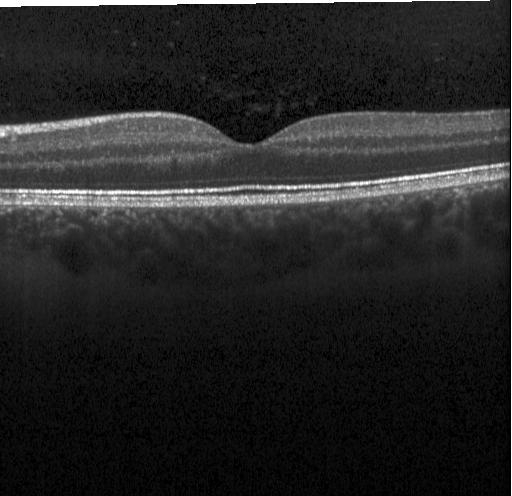
Heidelberg Spectralis; retinal OCT B-scan.
The scan shows neither choroidal neovascularization, diabetic macular edema, nor drusen.